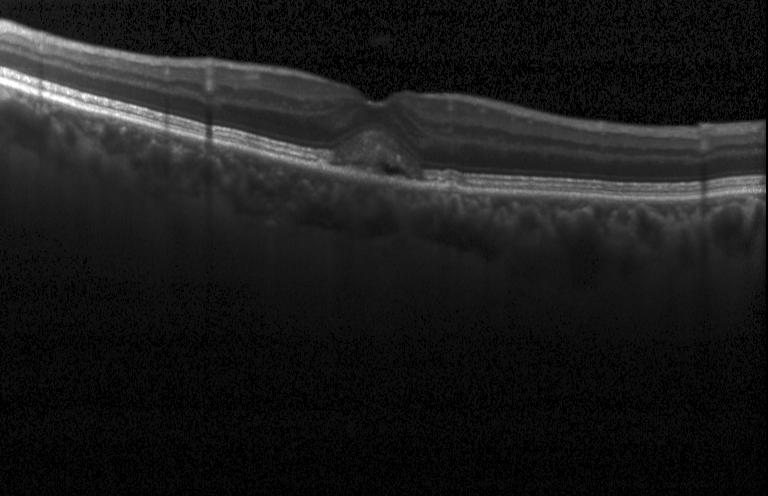 Diagnosis: a choroidal neovascular membrane.